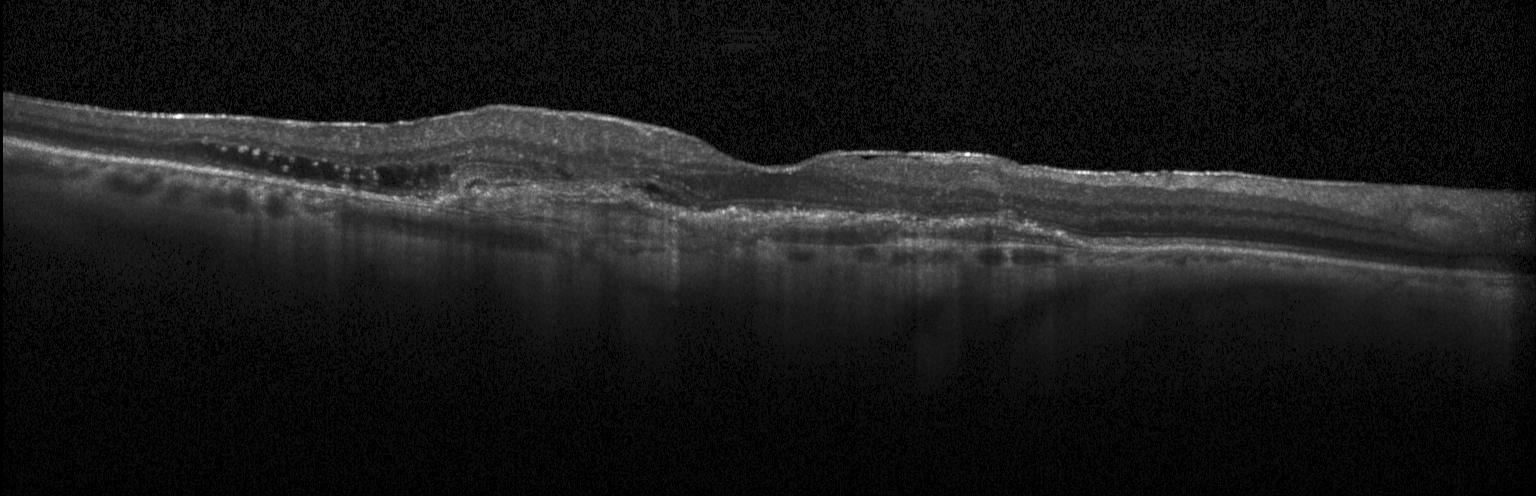

Dx: CNV.